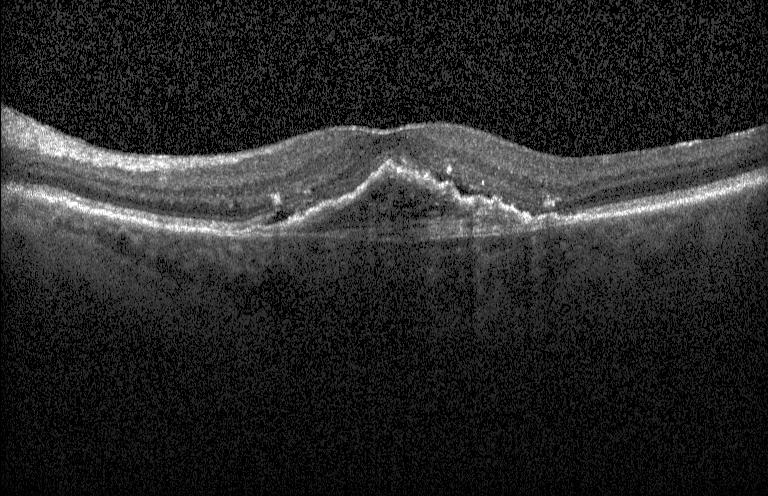

Optical coherence tomography scan. Finding: choroidal neovascularization.